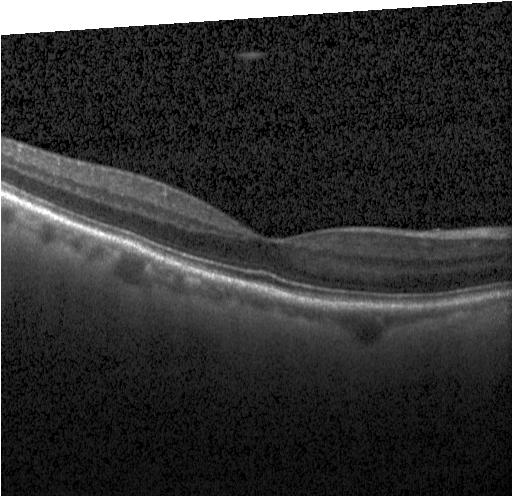
OCT line scan. Finding: neither choroidal neovascularization, diabetic macular edema, nor drusen.